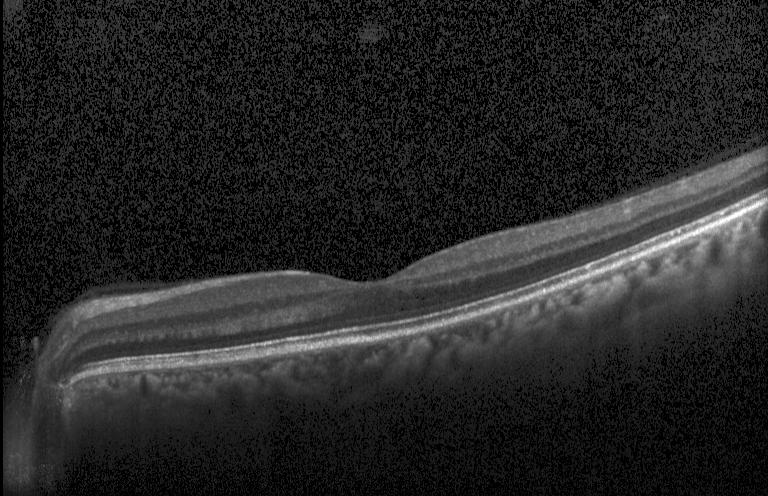

Spectral-domain optical coherence tomography, optical coherence tomography scan, Heidelberg Spectralis
Dx: neither choroidal neovascularization, diabetic macular edema, nor drusen.